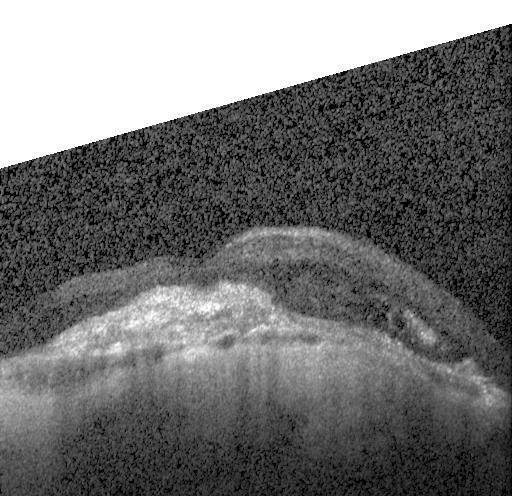
Acquired on a Heidelberg Spectralis · OCT line scan · horizontal scan through the fovea · spectral-domain optical coherence tomography. Finding: a choroidal neovascular membrane.